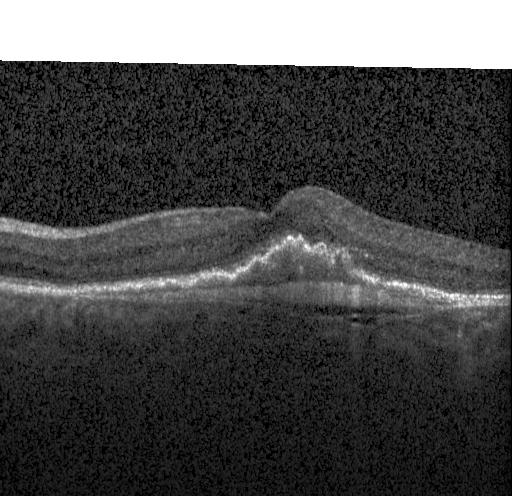 Spectral-domain optical coherence tomography · horizontal scan through the fovea · Heidelberg Spectralis OCT system · optical coherence tomography B-scan. Finding: a choroidal neovascular membrane.